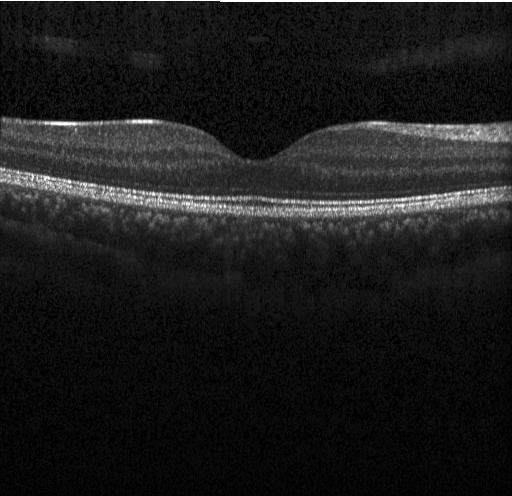

OCT line scan, spectral-domain optical coherence tomography, horizontal scan through the fovea, Heidelberg Spectralis.
Neither choroidal neovascularization, diabetic macular edema, nor drusen.